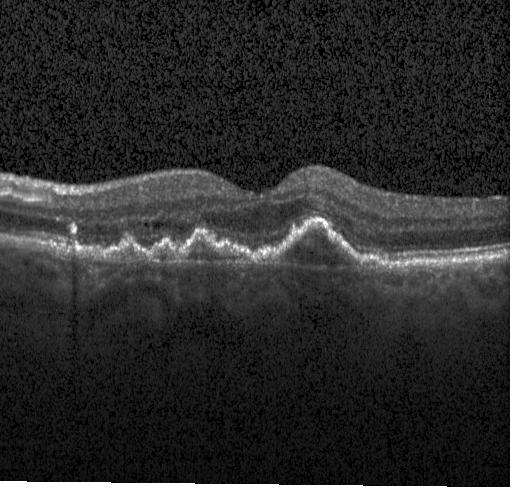

Acquired on a Heidelberg Spectralis, centered on the fovea, optical coherence tomography B-scan, SD-OCT — Impression: a choroidal neovascular membrane.